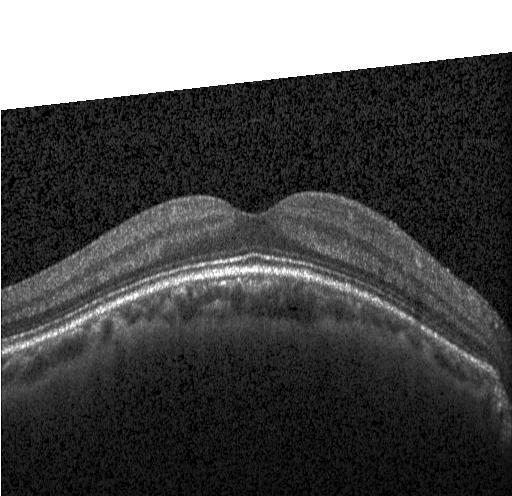
Heidelberg Spectralis · OCT line scan · horizontal scan through the fovea.
Macular OCT: neither choroidal neovascularization, diabetic macular edema, nor drusen.